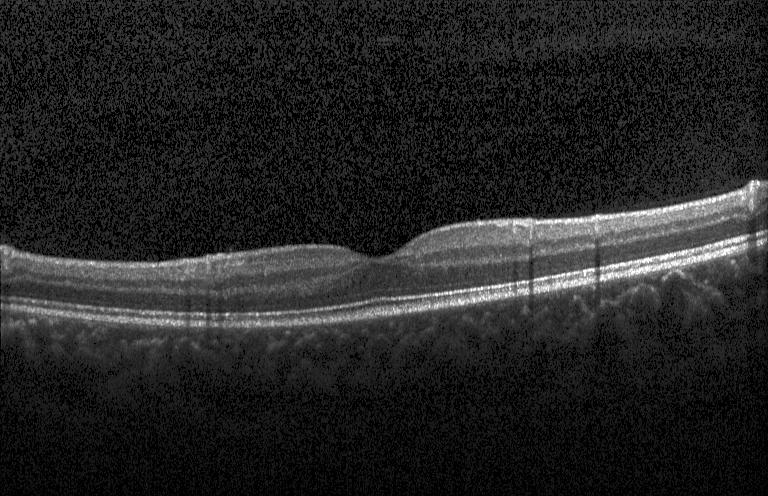 Retinal OCT cross-section. Assessment: no evidence of choroidal neovascularization, diabetic macular edema, or drusen.